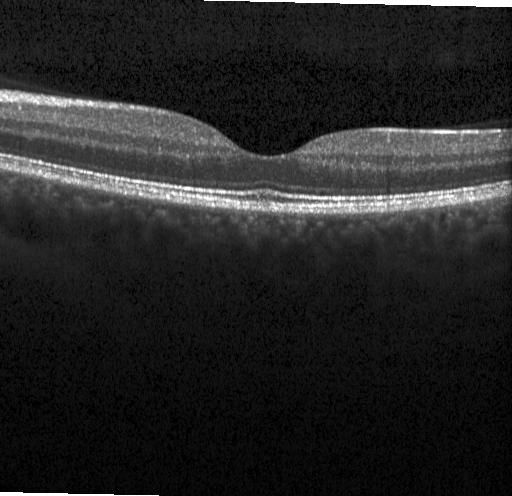

The scan shows no choroidal neovascularization, no diabetic macular edema, and no drusen.